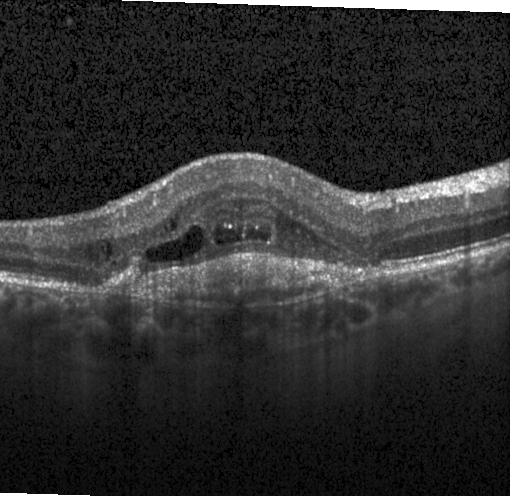
Assessment: a choroidal neovascular membrane.